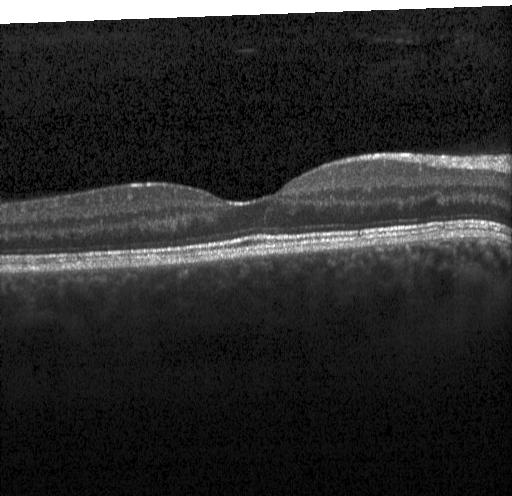 Finding: neither choroidal neovascularization, diabetic macular edema, nor drusen.